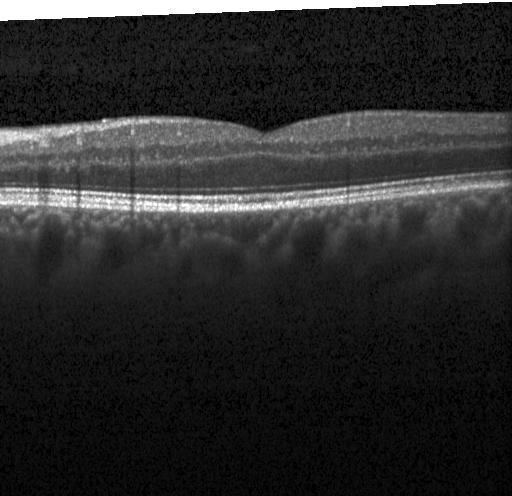

Instrument: Heidelberg Spectralis. Retinal OCT B-scan. This B-scan demonstrates no evidence of choroidal neovascularization, diabetic macular edema, or drusen.